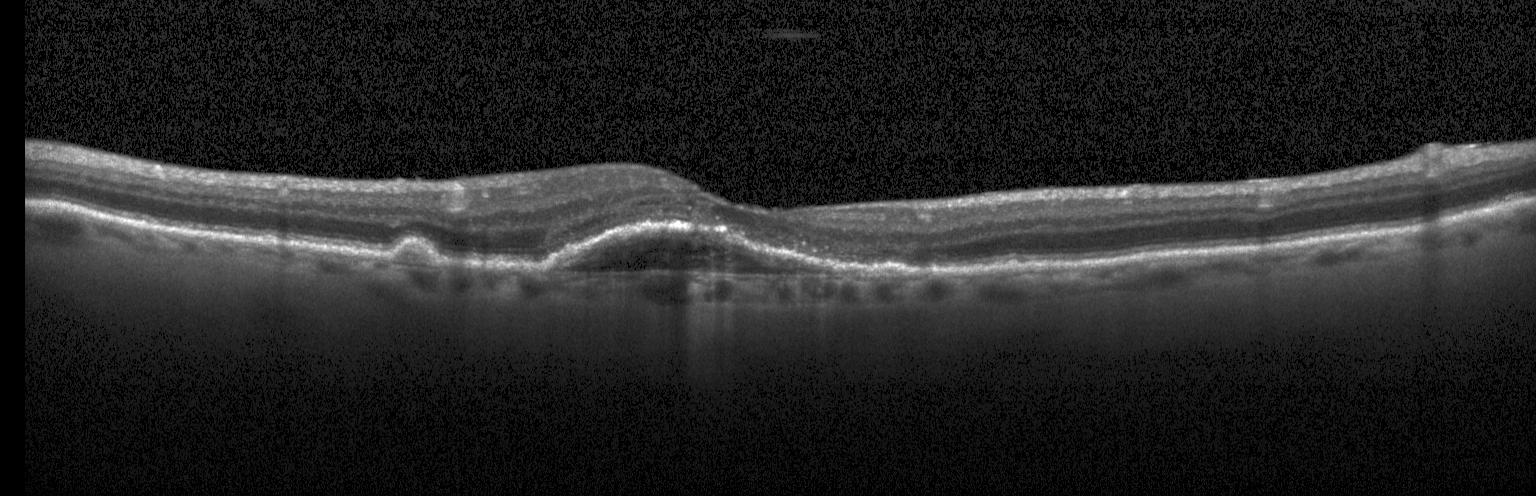

Diagnosis: CNV.